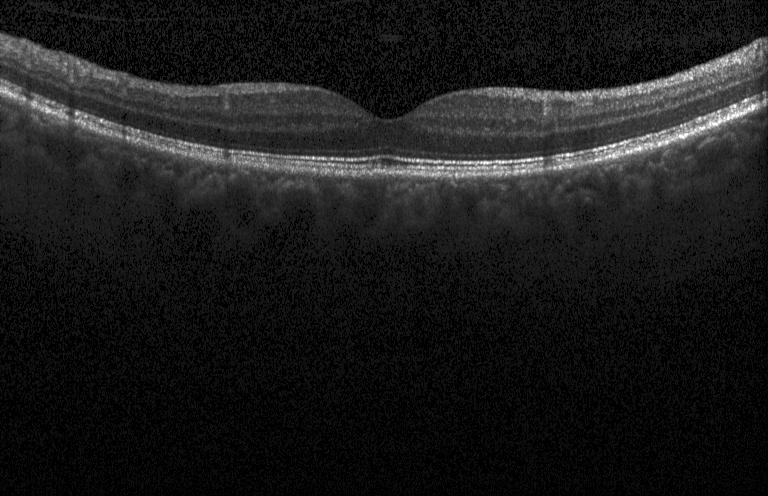 Diagnosis: no choroidal neovascularization, no diabetic macular edema, and no drusen.